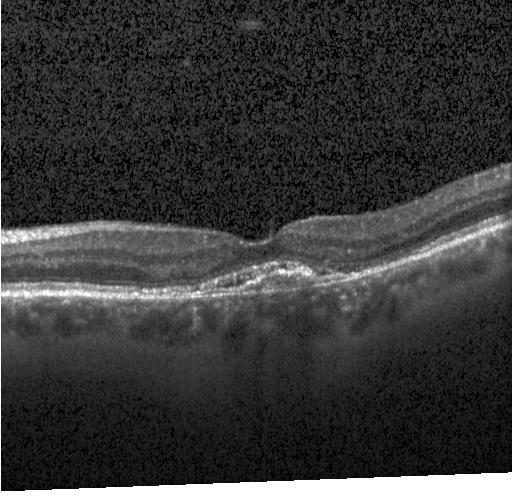

OCT B-scan · Heidelberg Spectralis OCT system · SD-OCT.
Diagnosis: choroidal neovascularization (CNV).